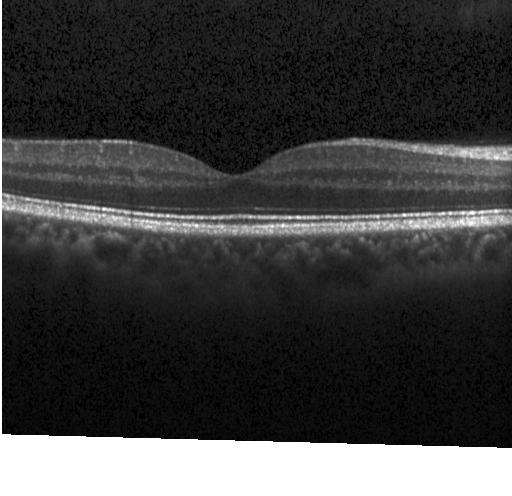
Retinal OCT B-scan · SD-OCT · macular scan · acquired on a Heidelberg Spectralis.
Finding: no choroidal neovascularization, diabetic macular edema, or drusen.